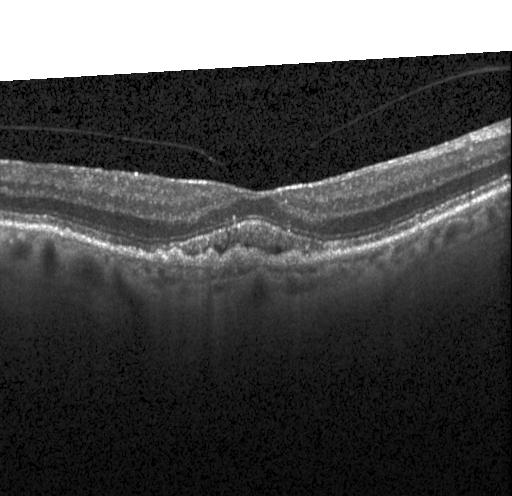 Finding: a choroidal neovascular membrane.